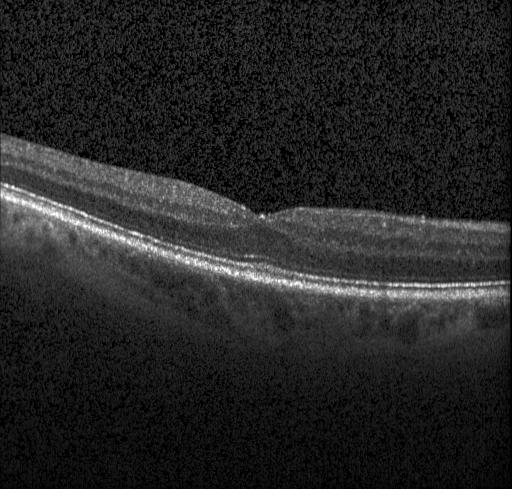
OCT B-scan.
Impression: no evidence of CNV, DME, or drusen.